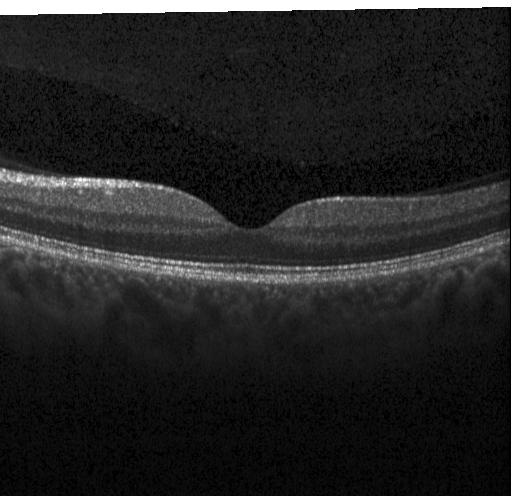 Diagnosis: no choroidal neovascularization, diabetic macular edema, or drusen.